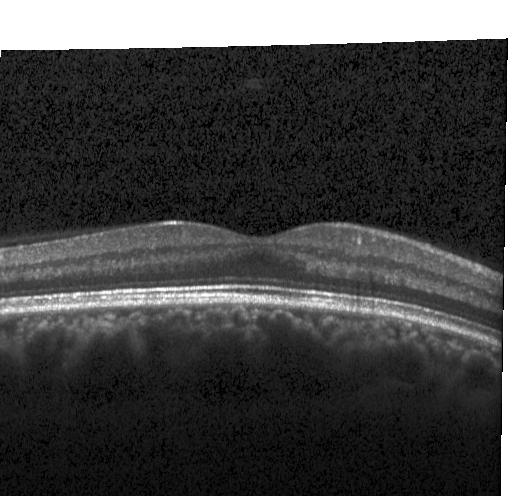

Finding: no CNV, DME, or drusen.